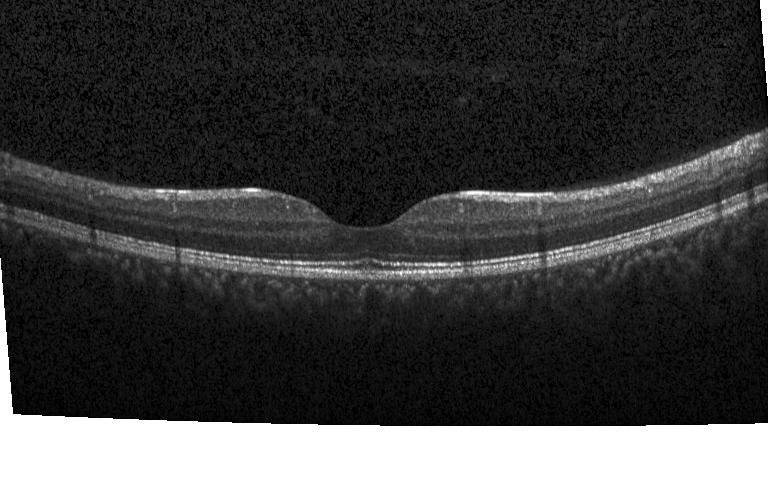

Diagnosis: no choroidal neovascularization, no diabetic macular edema, and no drusen.